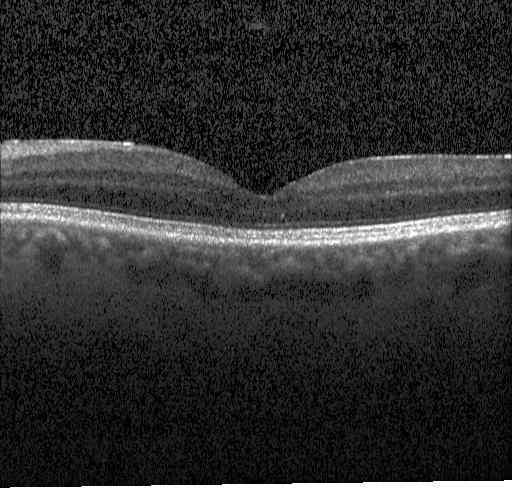 Macular scan. Retinal OCT cross-section. Acquired on a Heidelberg Spectralis.
Diagnosis: no CNV, no DME, and no drusen.